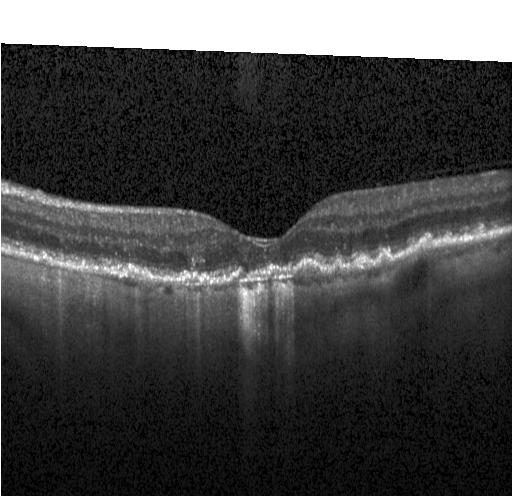 Horizontal scan through the fovea, instrument: Heidelberg Spectralis, spectral-domain optical coherence tomography, optical coherence tomography scan
Diagnosis: multiple drusen.